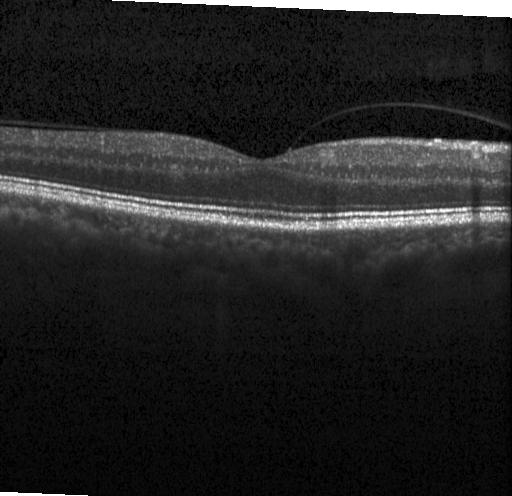 Retinal OCT B-scan.
The scan shows no choroidal neovascularization, no diabetic macular edema, and no drusen.